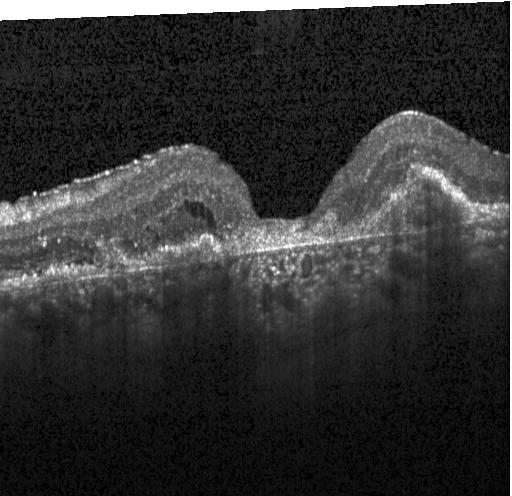 Diagnosis: CNV.